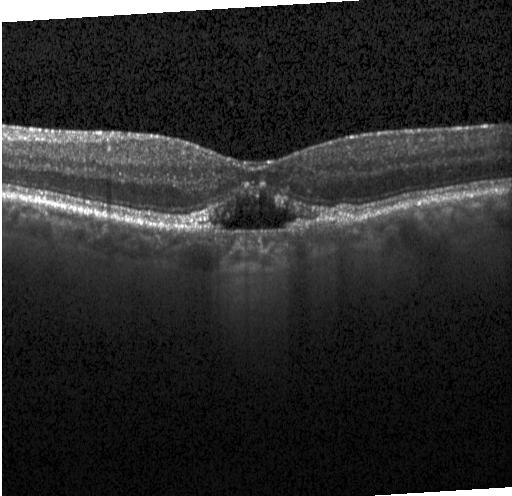 Retinal OCT cross-section. Macular scan
Assessment: choroidal neovascularization (CNV).